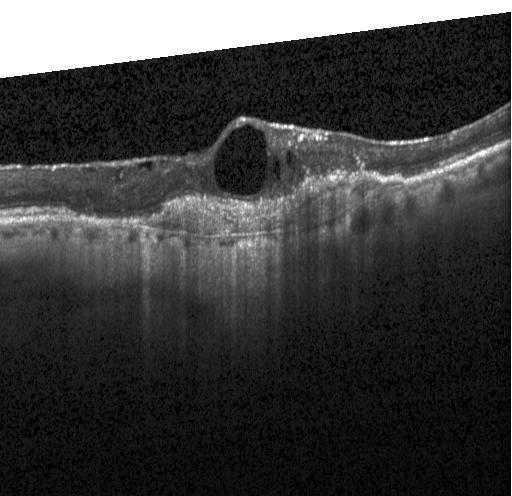
Optical coherence tomography scan
Dx: choroidal neovascularization.